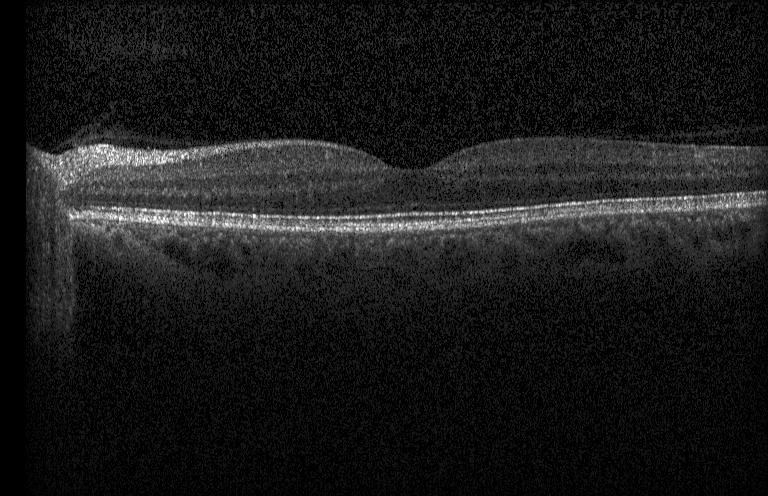 Macular OCT: no choroidal neovascularization, diabetic macular edema, or drusen.